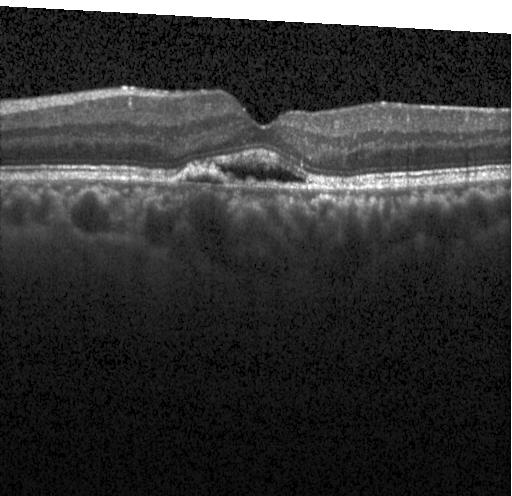 OCT line scan. SD-OCT. Impression: CNV.